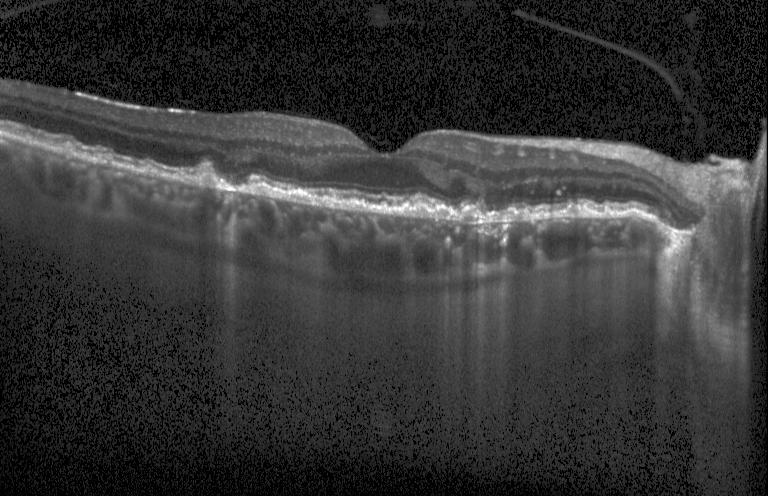 OCT scan showing multiple drusen.